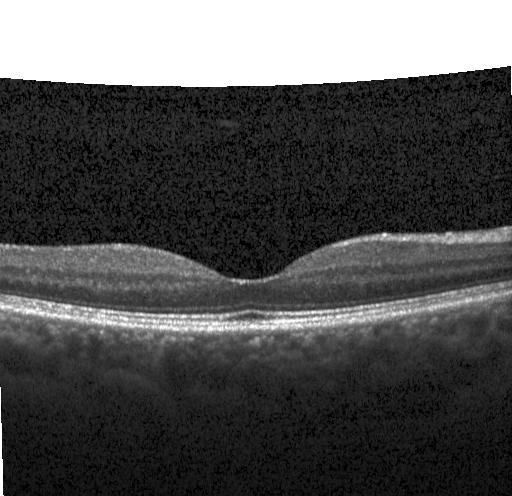
OCT B-scan showing no CNV, DME, or drusen.